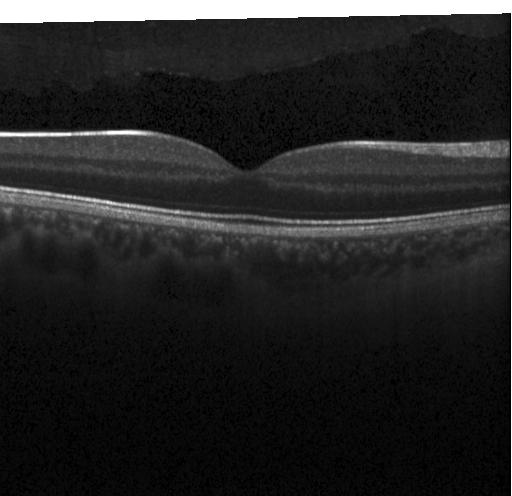 OCT finding: no choroidal neovascularization, no diabetic macular edema, and no drusen.